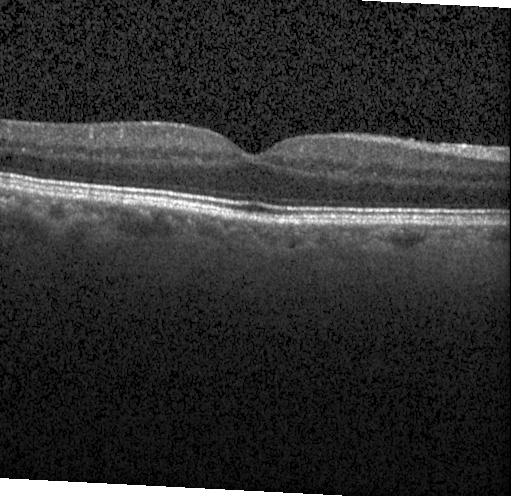

OCT B-scan; through the macula; Heidelberg Spectralis OCT system
Finding: neither choroidal neovascularization, diabetic macular edema, nor drusen.